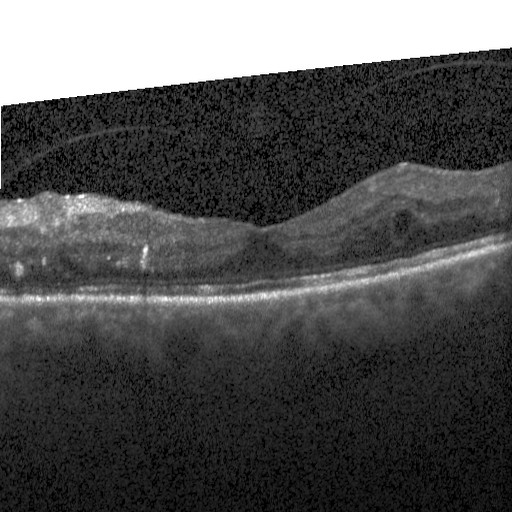 Spectral-domain optical coherence tomography; horizontal scan through the fovea; OCT B-scan; Heidelberg Spectralis OCT system.
Impression: DME.